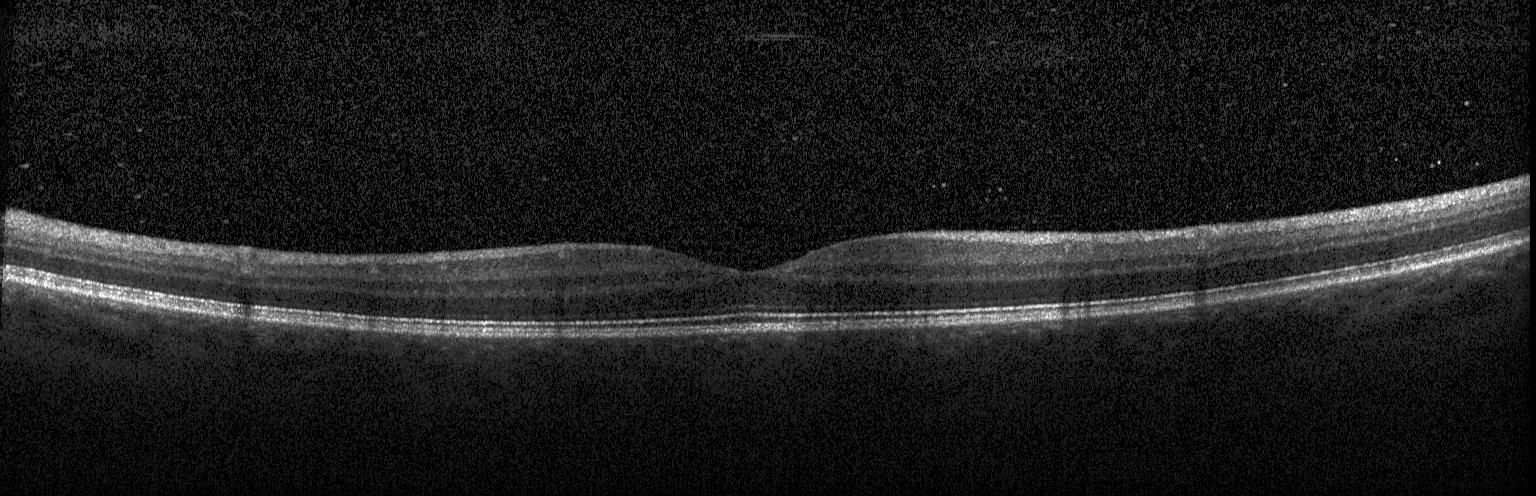 OCT B-scan.
The scan shows no CNV, DME, or drusen.